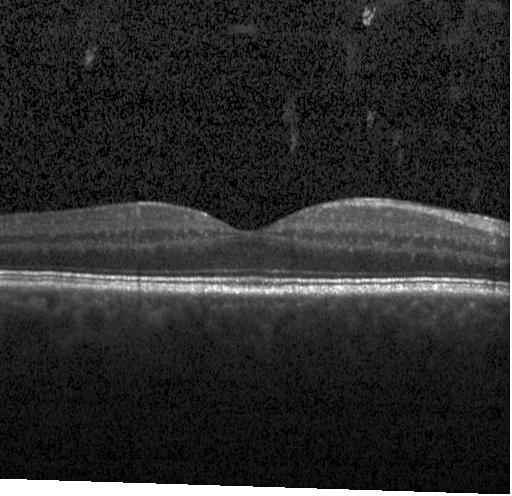

OCT finding: no evidence of choroidal neovascularization, diabetic macular edema, or drusen.